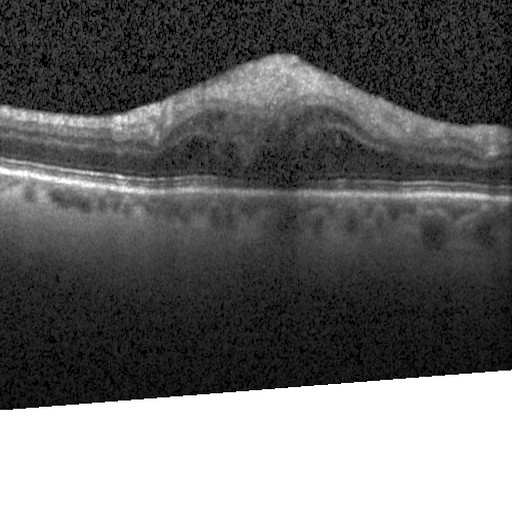

OCT B-scan.
This B-scan demonstrates diabetic macular edema (DME).